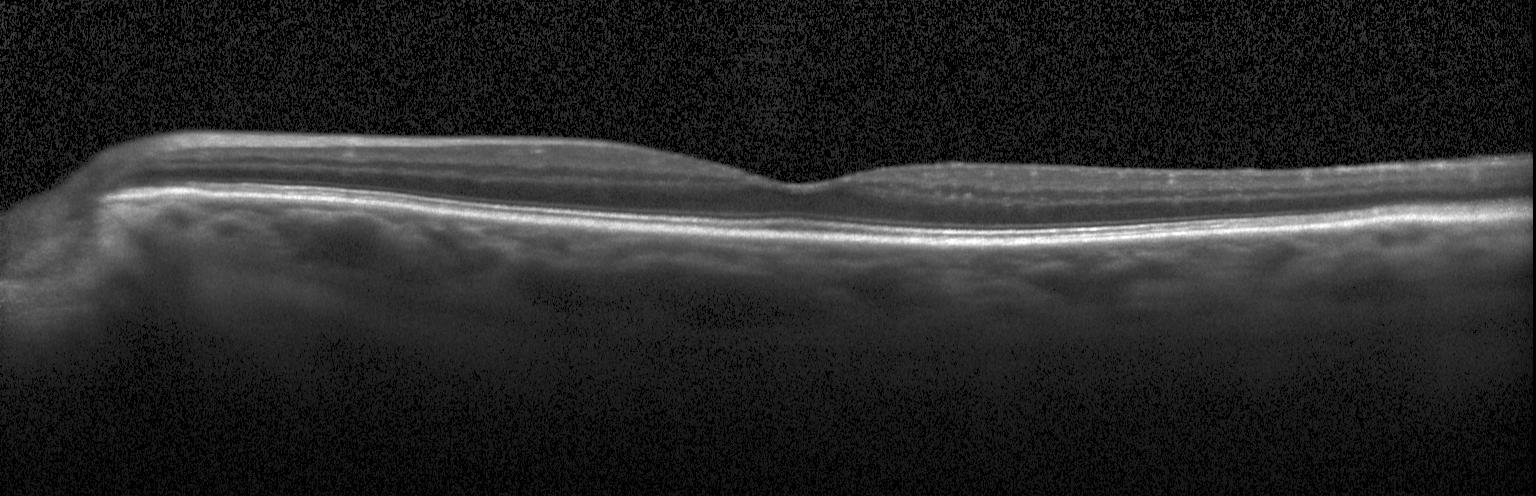
Heidelberg Spectralis OCT system · spectral-domain OCT · retinal OCT B-scan.
This B-scan demonstrates no evidence of choroidal neovascularization, diabetic macular edema, or drusen.